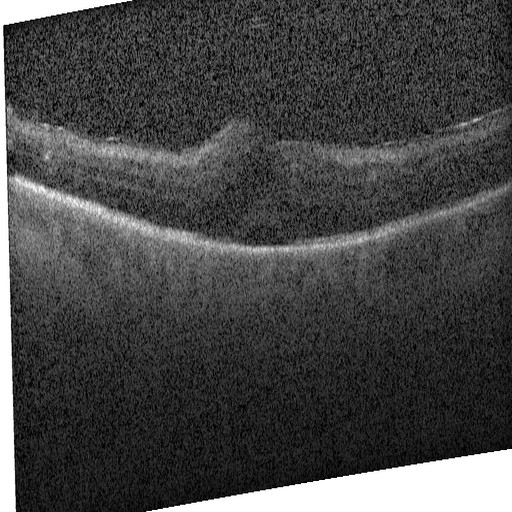

Impression: diabetic macular edema.